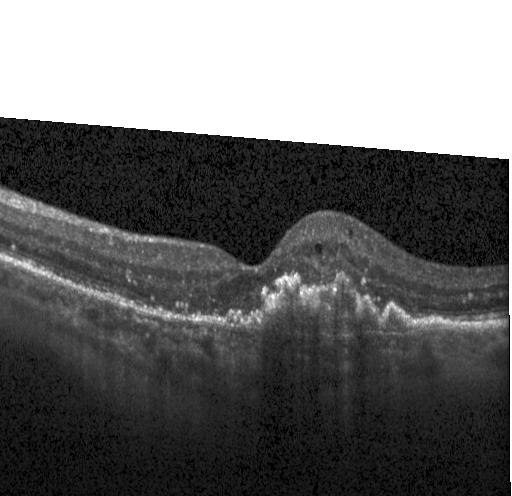 Horizontal scan through the fovea. Optical coherence tomography scan
Dx: CNV.